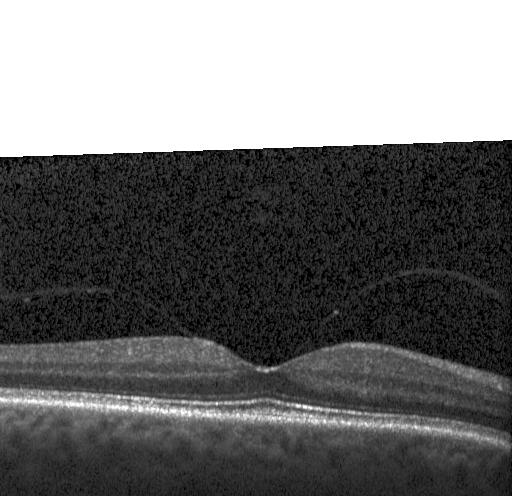
Macular OCT: no evidence of choroidal neovascularization, diabetic macular edema, or drusen.